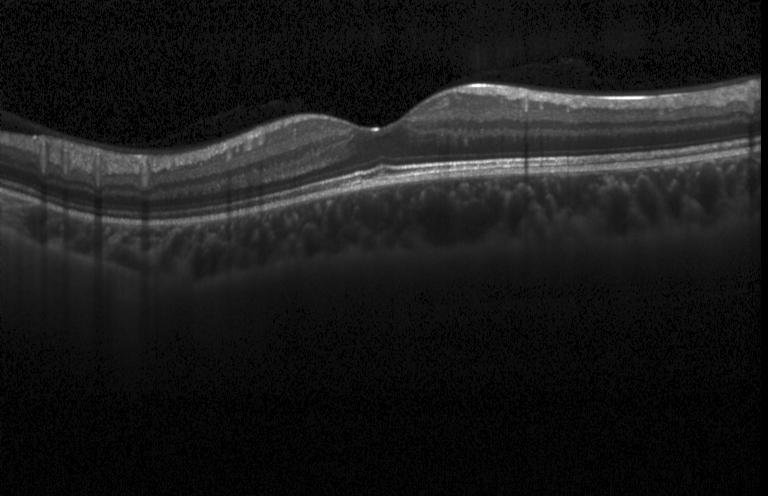 Heidelberg Spectralis · SD-OCT · OCT line scan · centered on the fovea. Diagnosis: no evidence of CNV, DME, or drusen.